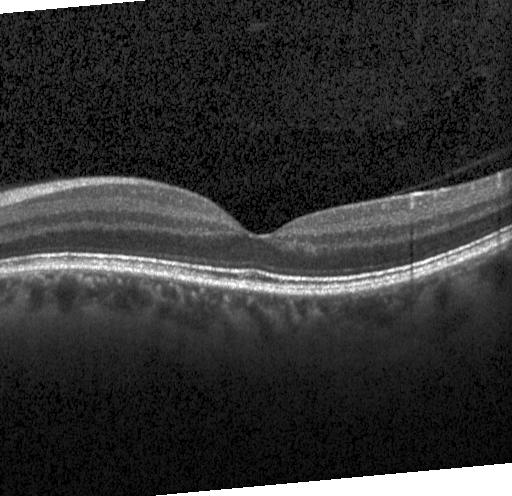

Finding: no evidence of choroidal neovascularization, diabetic macular edema, or drusen.